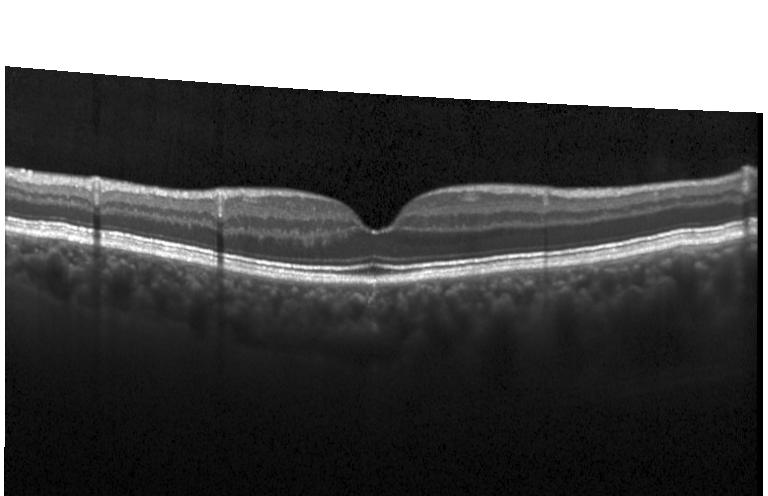
Spectral-domain OCT. Optical coherence tomography B-scan. Acquired on a Heidelberg Spectralis. Fovea-centered. The scan shows neither choroidal neovascularization, diabetic macular edema, nor drusen.